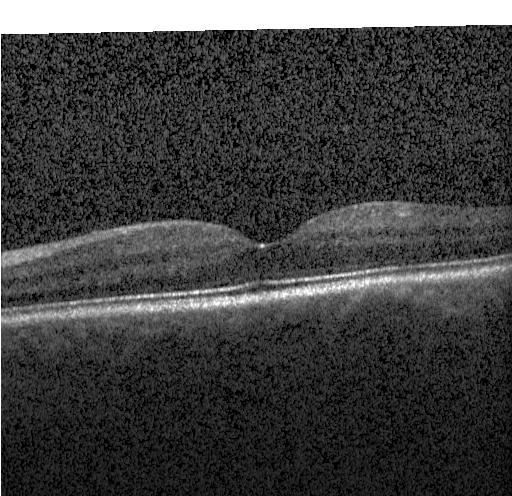 Instrument: Heidelberg Spectralis · optical coherence tomography B-scan · spectral-domain optical coherence tomography. Finding: no choroidal neovascularization, diabetic macular edema, or drusen.